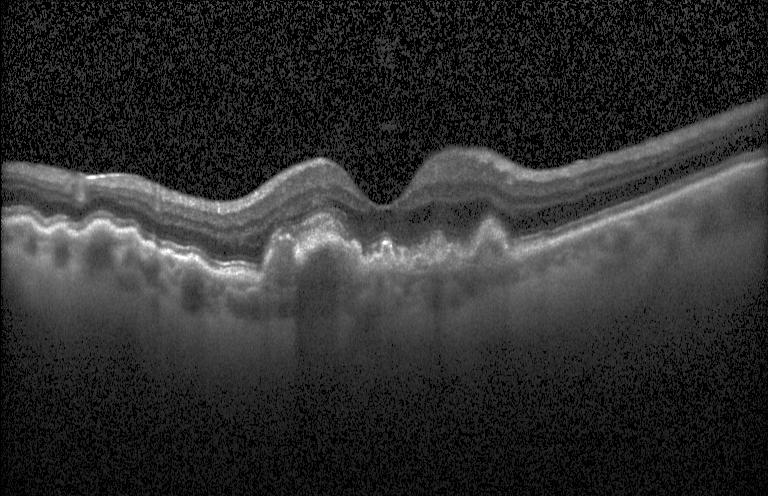
SD-OCT, retinal OCT cross-section — Diagnosis: a choroidal neovascular membrane.